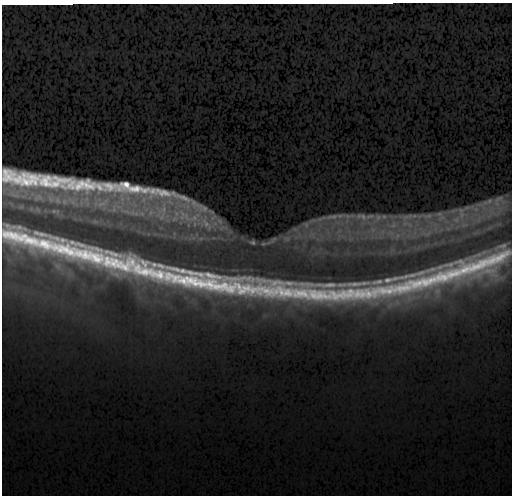

Spectral-domain OCT, macular scan, retinal OCT B-scan — Diagnosis: multiple drusen.